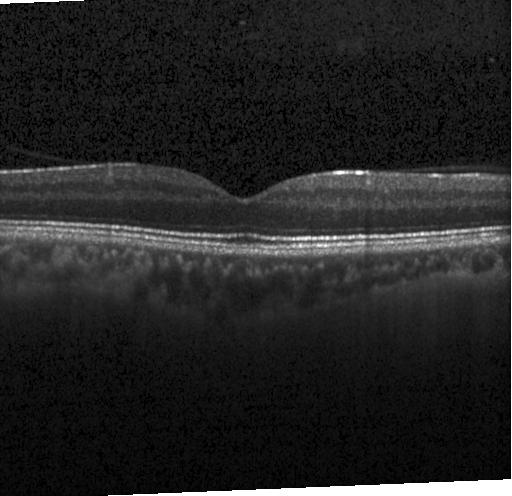
OCT line scan — Diagnosis: neither choroidal neovascularization, diabetic macular edema, nor drusen.